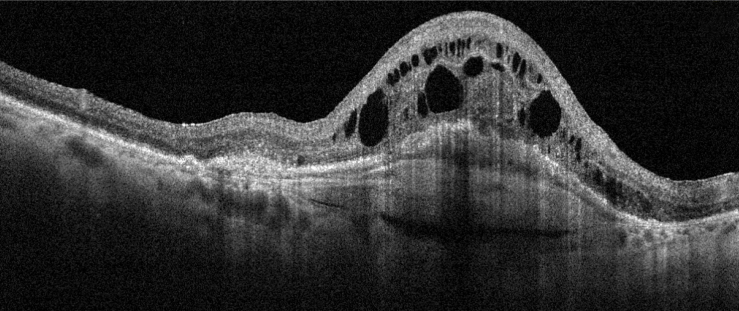

Fovea-centered · OCT B-scan · Optovue Avanti RTVue XR.
Dx: AMD.